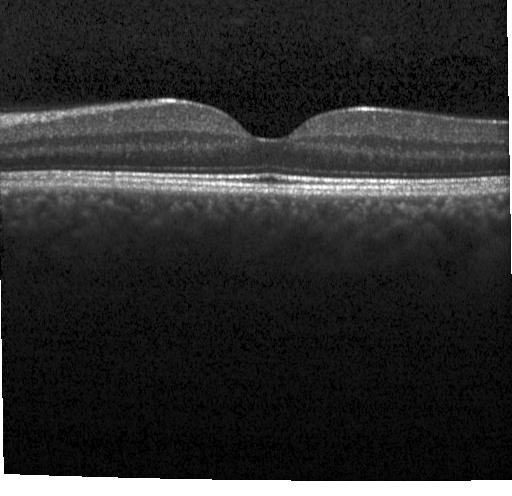
Heidelberg Spectralis; macular scan; OCT line scan; spectral-domain optical coherence tomography.
No evidence of CNV, DME, or drusen.